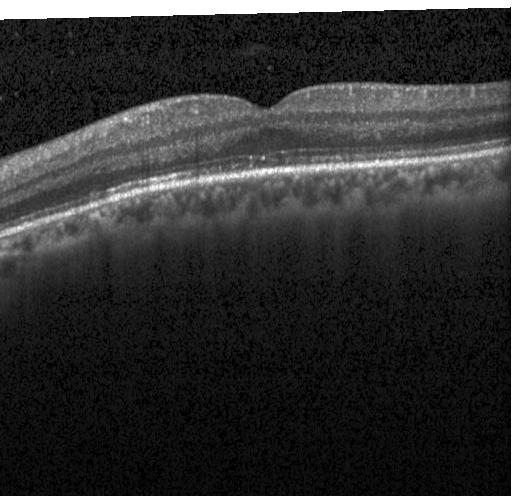
SD-OCT. Optical coherence tomography scan. Horizontal scan through the fovea. Heidelberg Spectralis OCT system. The scan shows no choroidal neovascularization, no diabetic macular edema, and no drusen.